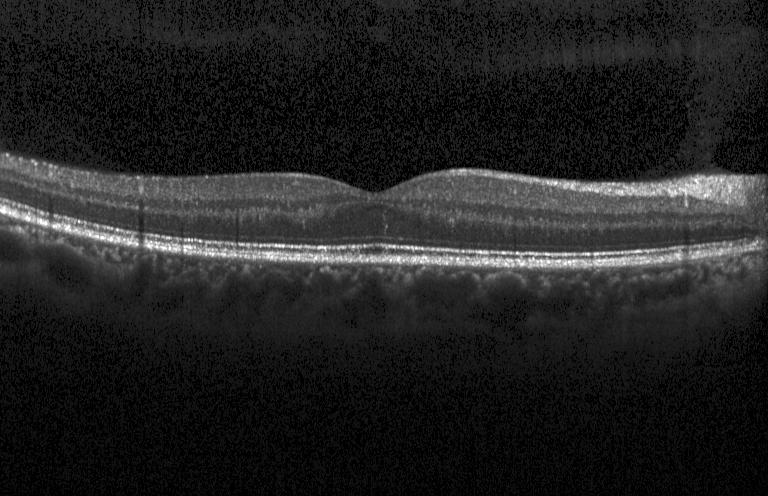 Fovea-centered · spectral-domain optical coherence tomography · optical coherence tomography B-scan · Heidelberg Spectralis. Diagnosis: no choroidal neovascularization, no diabetic macular edema, and no drusen.